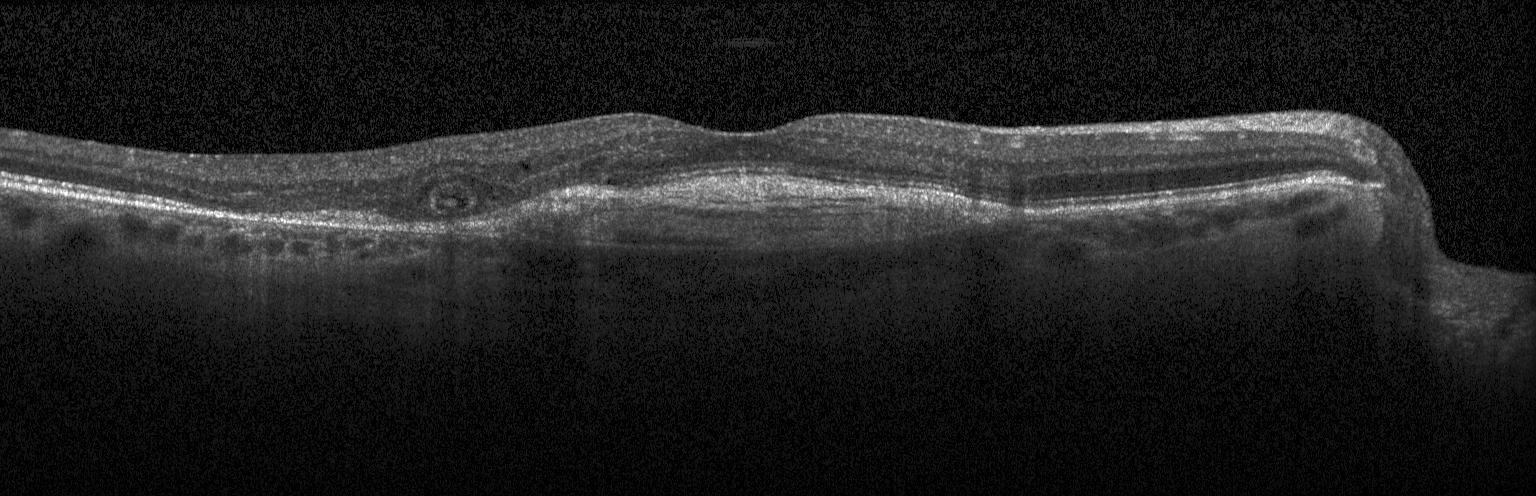
Spectral-domain optical coherence tomography, retinal OCT B-scan, centered on the fovea, Heidelberg Spectralis — Impression: choroidal neovascularization.